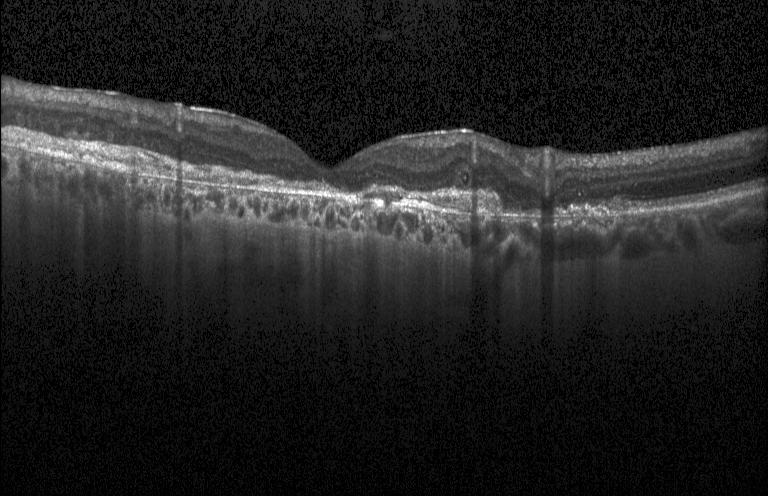

Retinal OCT B-scan.
Finding: a choroidal neovascular membrane.